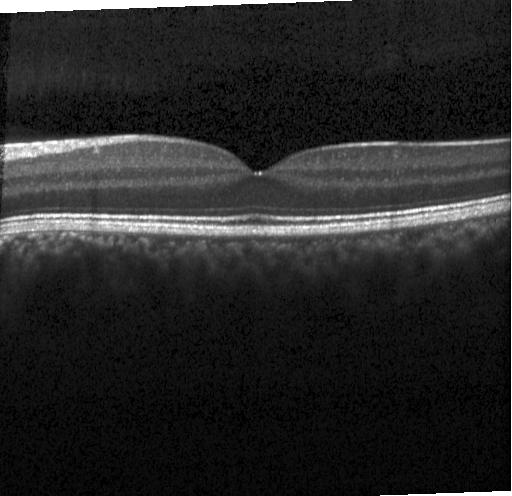
No choroidal neovascularization, diabetic macular edema, or drusen.